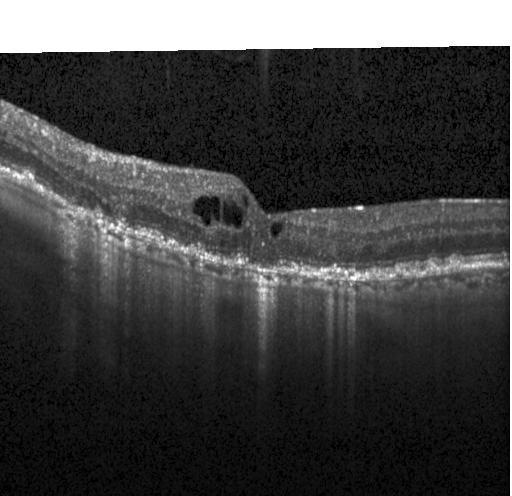
OCT B-scan. Fovea-centered. Finding: a choroidal neovascular membrane.